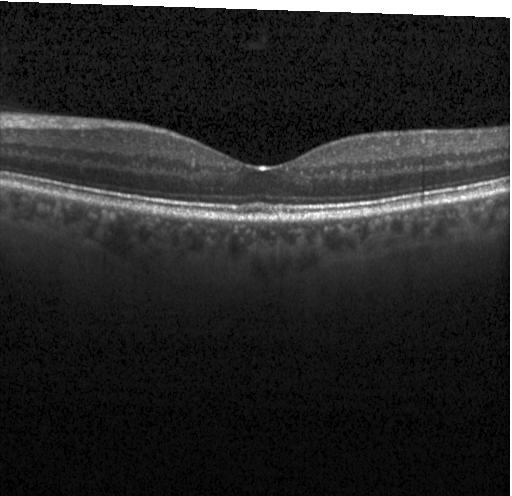

Macular scan, optical coherence tomography B-scan, spectral-domain optical coherence tomography.
Finding: no choroidal neovascularization, diabetic macular edema, or drusen.